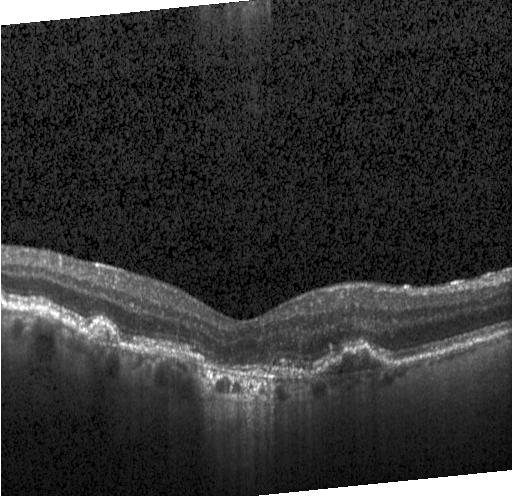 Through the macula. OCT line scan — Impression: a choroidal neovascular membrane.